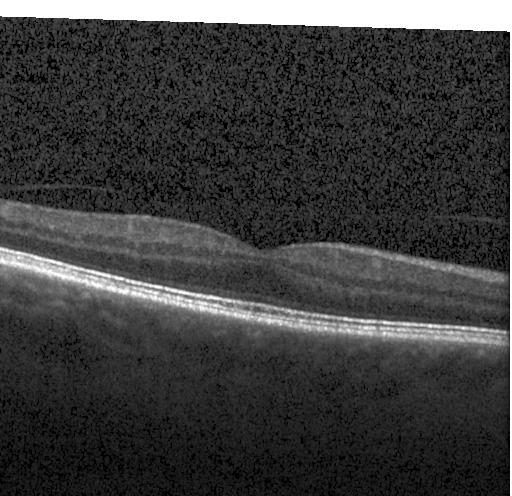

Dx: no choroidal neovascularization, no diabetic macular edema, and no drusen.